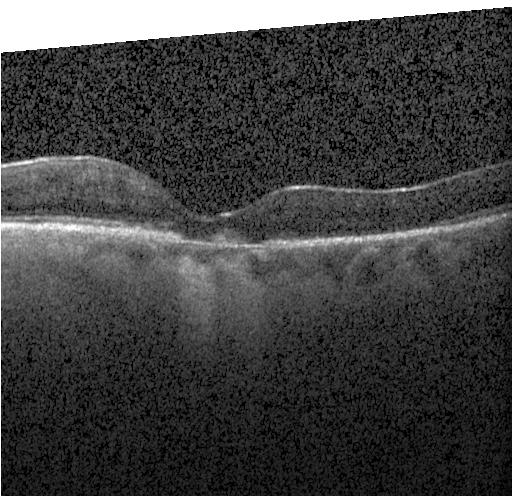
This B-scan demonstrates choroidal neovascularization.